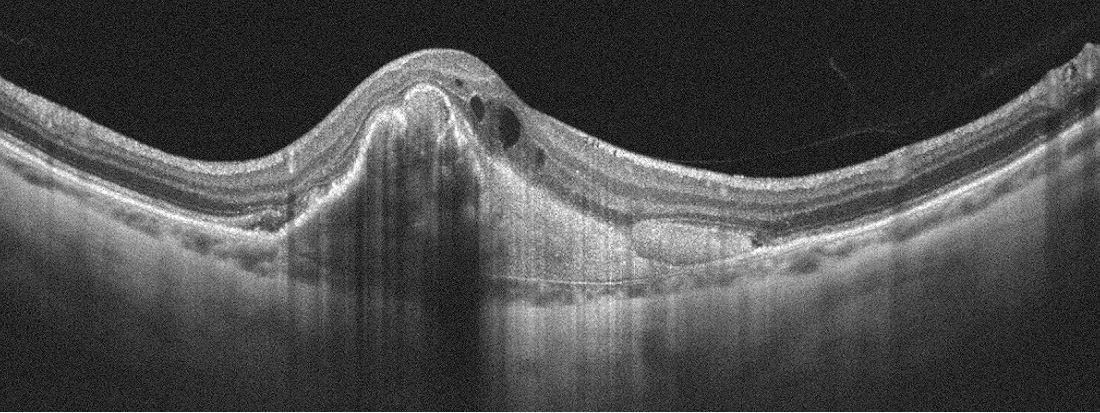 Optovue Avanti RTVue XR; OCT B-scan
Impression: AMD.